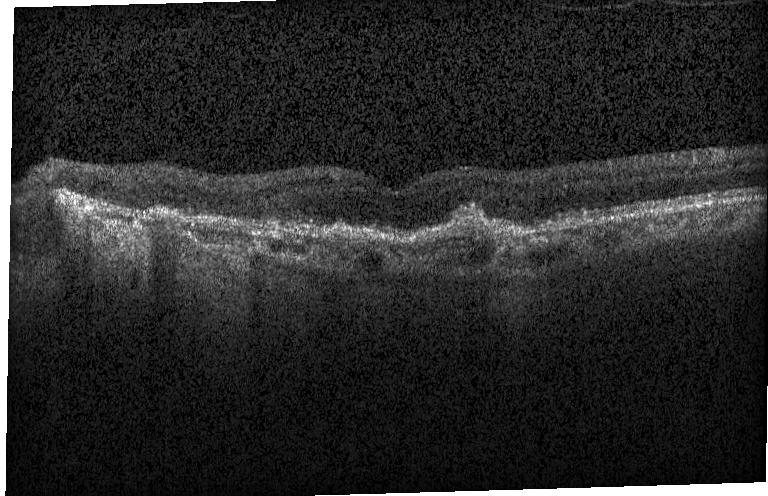
Optical coherence tomography B-scan · SD-OCT · macular scan — The scan shows CNV.